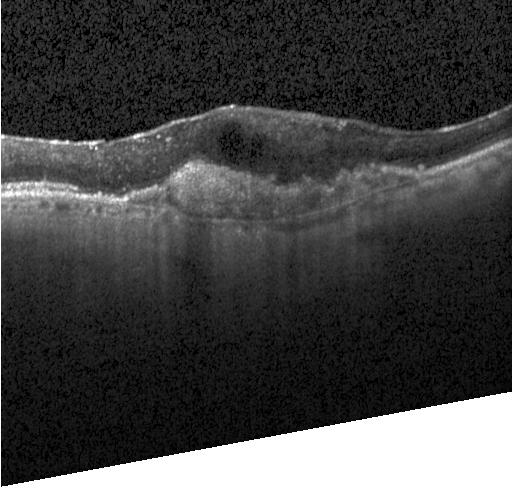

Choroidal neovascularization (CNV).